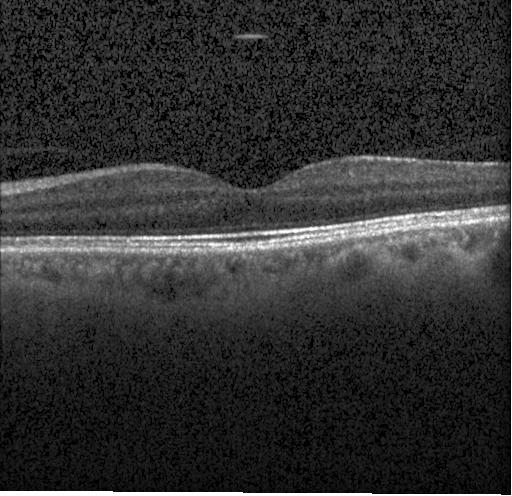 OCT finding: no CNV, DME, or drusen.